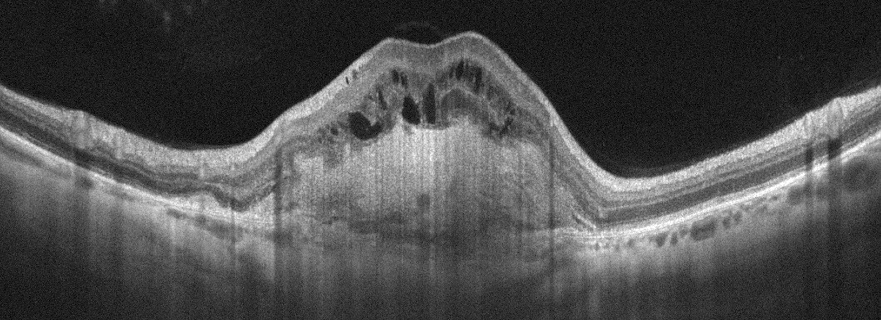
Macular scan; OCT line scan — Diagnosis: AMD.